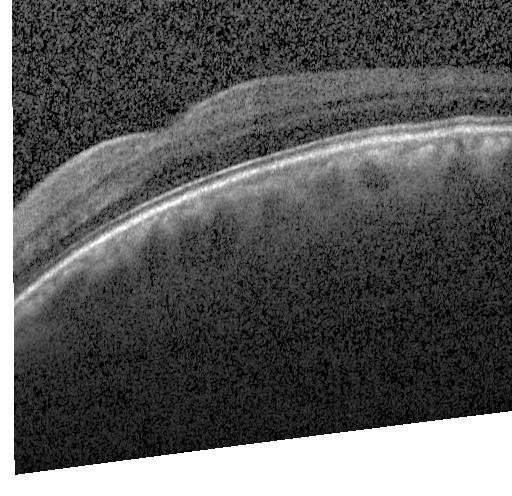
Optical coherence tomography scan
This B-scan demonstrates no choroidal neovascularization, no diabetic macular edema, and no drusen.